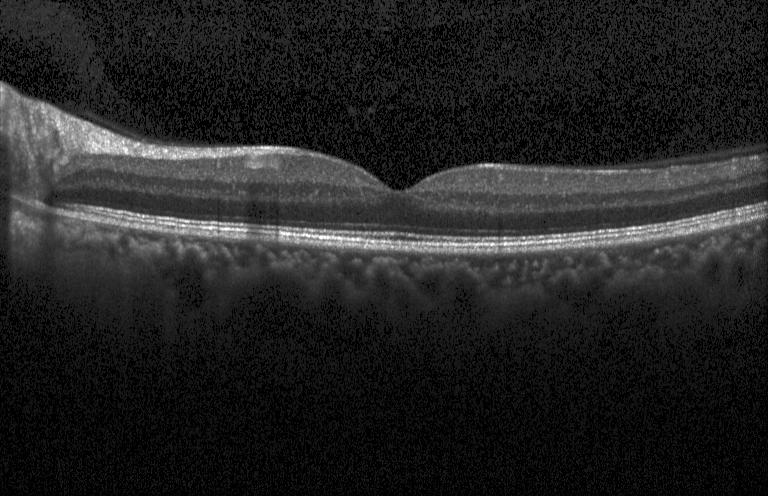 Retinal OCT cross-section. This B-scan demonstrates no evidence of choroidal neovascularization, diabetic macular edema, or drusen.